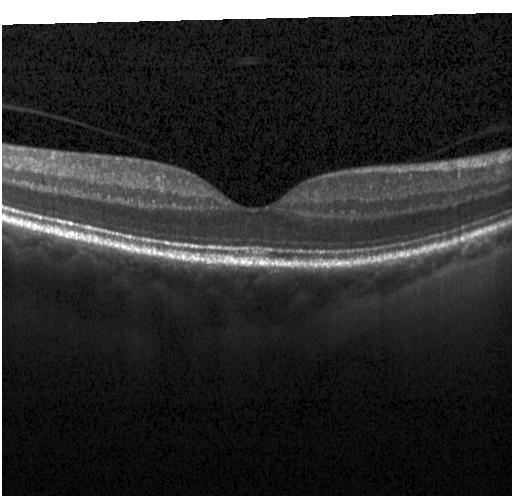 Horizontal scan through the fovea. Optical coherence tomography B-scan — The scan shows no choroidal neovascularization, diabetic macular edema, or drusen.